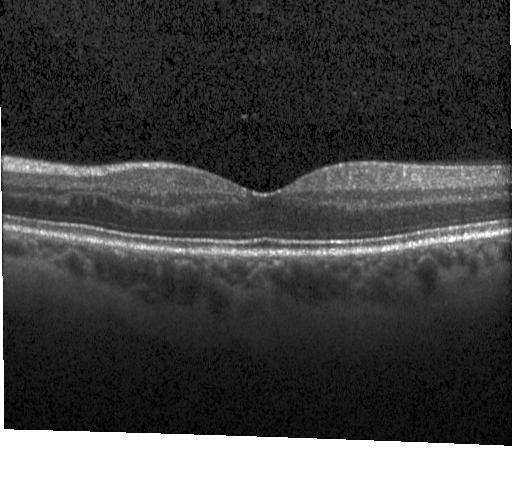 Macular scan, Heidelberg Spectralis, SD-OCT, OCT line scan
No choroidal neovascularization, diabetic macular edema, or drusen.